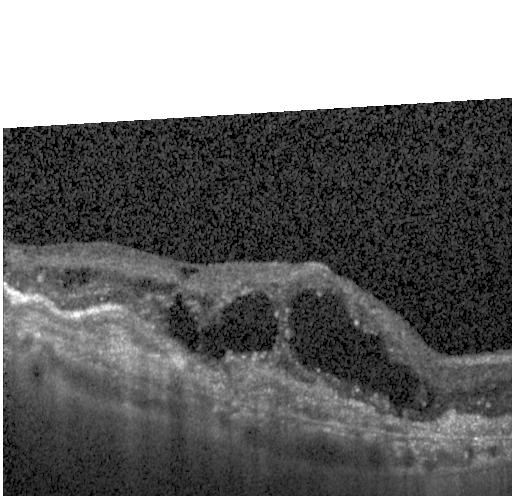
OCT line scan · acquired on a Heidelberg Spectralis.
The scan shows a choroidal neovascular membrane.